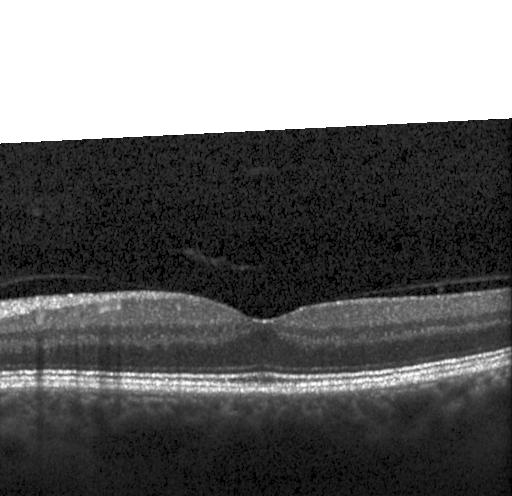 Finding: no choroidal neovascularization, no diabetic macular edema, and no drusen.